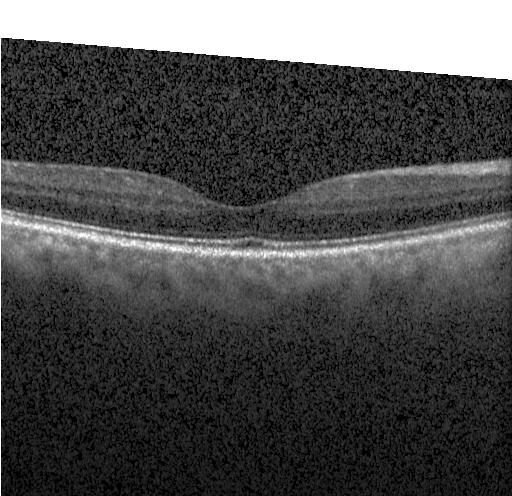
Finding: neither CNV, DME, nor drusen.